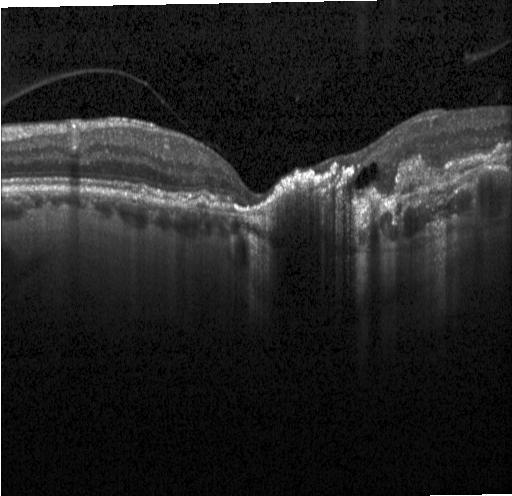
SD-OCT; horizontal scan through the fovea; retinal OCT cross-section.
Finding: a choroidal neovascular membrane.